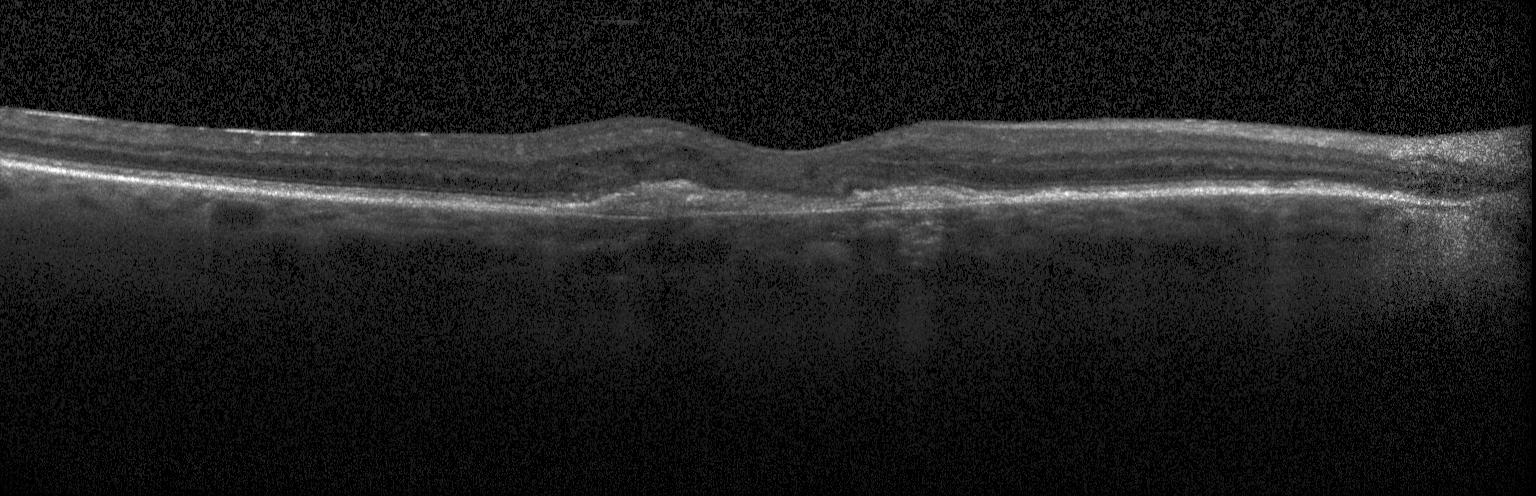 Diagnosis: CNV.